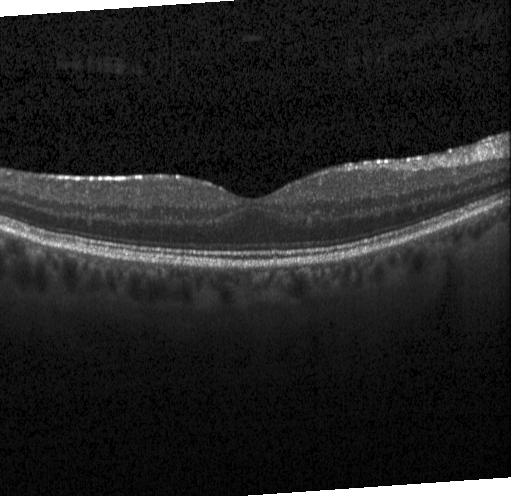
OCT line scan; macular scan — The scan shows neither CNV, DME, nor drusen.